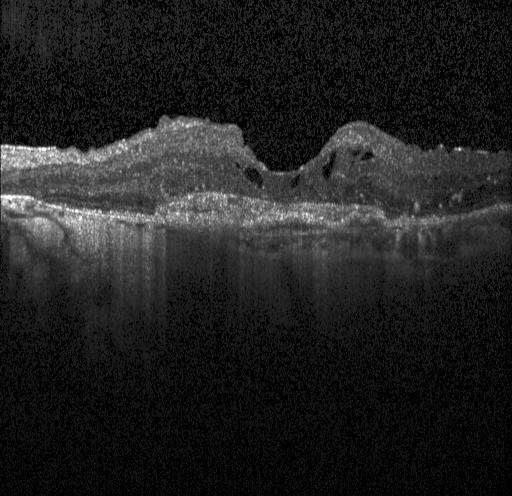

Optical coherence tomography B-scan — Diagnosis: a choroidal neovascular membrane.